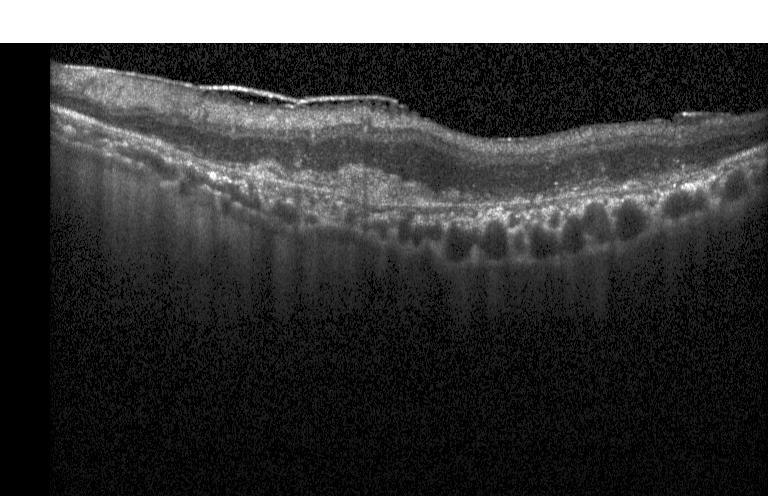 Fovea-centered, retinal OCT cross-section — Assessment: a choroidal neovascular membrane.